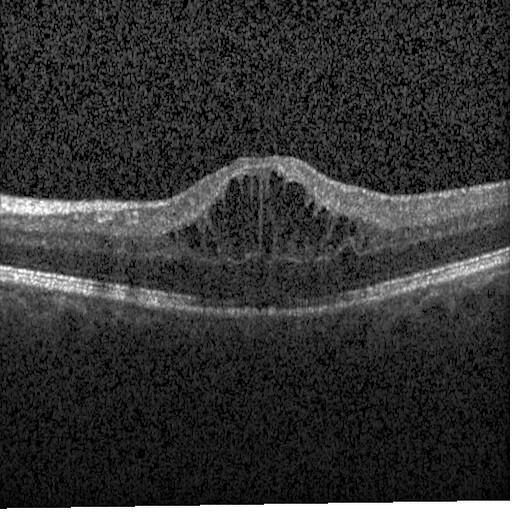

Retinal OCT B-scan. Finding: diabetic macular edema.